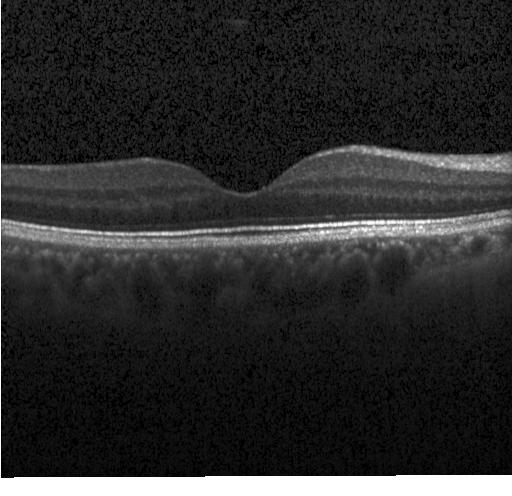
OCT line scan. Diagnosis: neither CNV, DME, nor drusen.